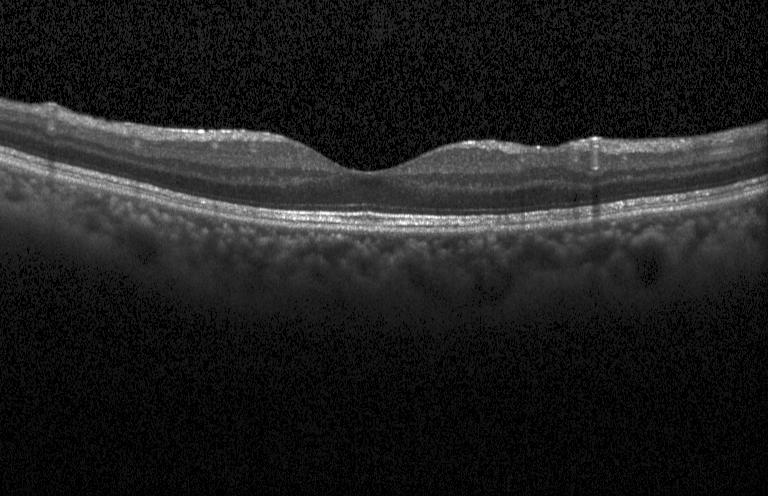

Centered on the fovea; optical coherence tomography B-scan — Diagnosis: neither CNV, DME, nor drusen.